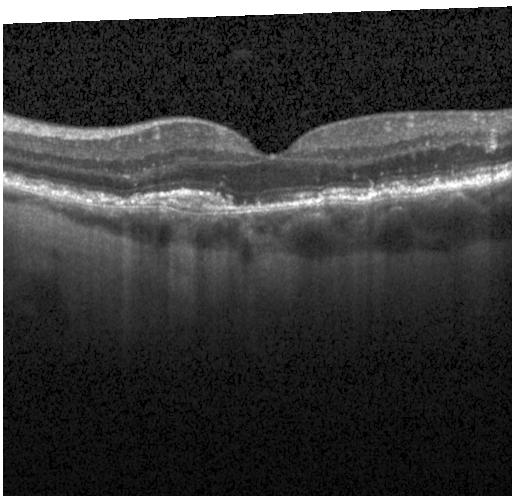 Spectral-domain OCT. Optical coherence tomography scan. Fovea-centered — Assessment: a choroidal neovascular membrane.